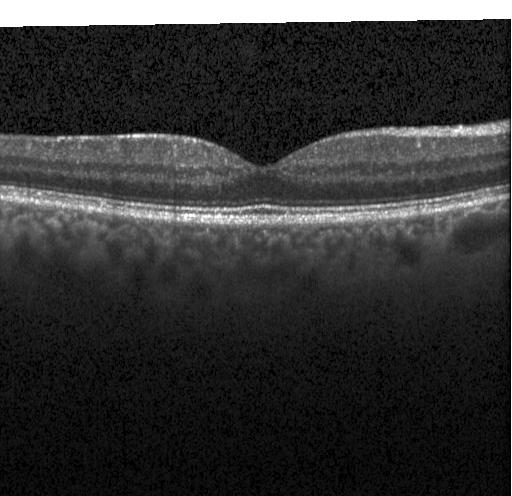

Spectral-domain OCT. OCT B-scan. Macular scan. Instrument: Heidelberg Spectralis. Dx: no choroidal neovascularization, no diabetic macular edema, and no drusen.